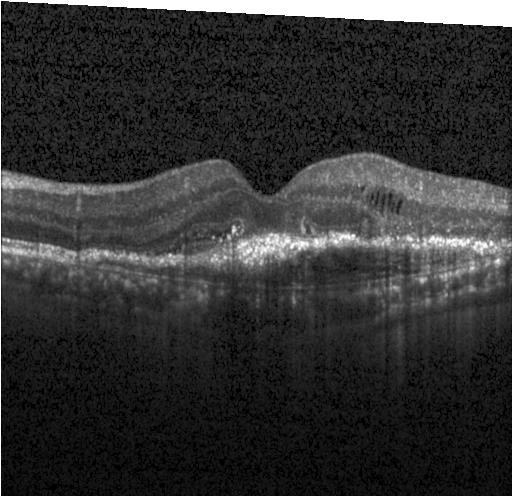 This B-scan demonstrates a choroidal neovascular membrane.